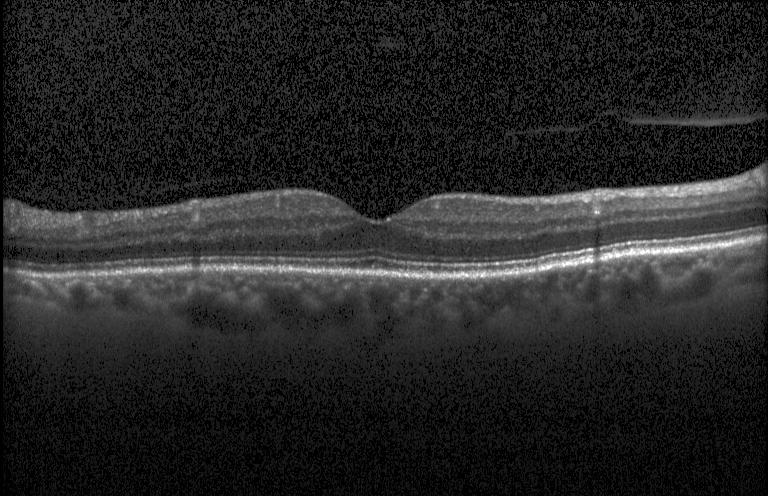
Retinal OCT B-scan. Spectral-domain OCT.
Impression: no evidence of choroidal neovascularization, diabetic macular edema, or drusen.